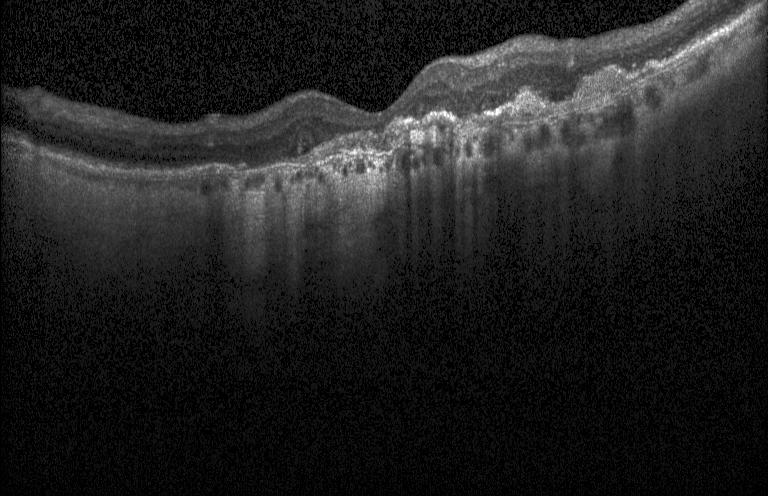

Retinal OCT B-scan · acquired on a Heidelberg Spectralis. This B-scan demonstrates choroidal neovascularization (CNV).